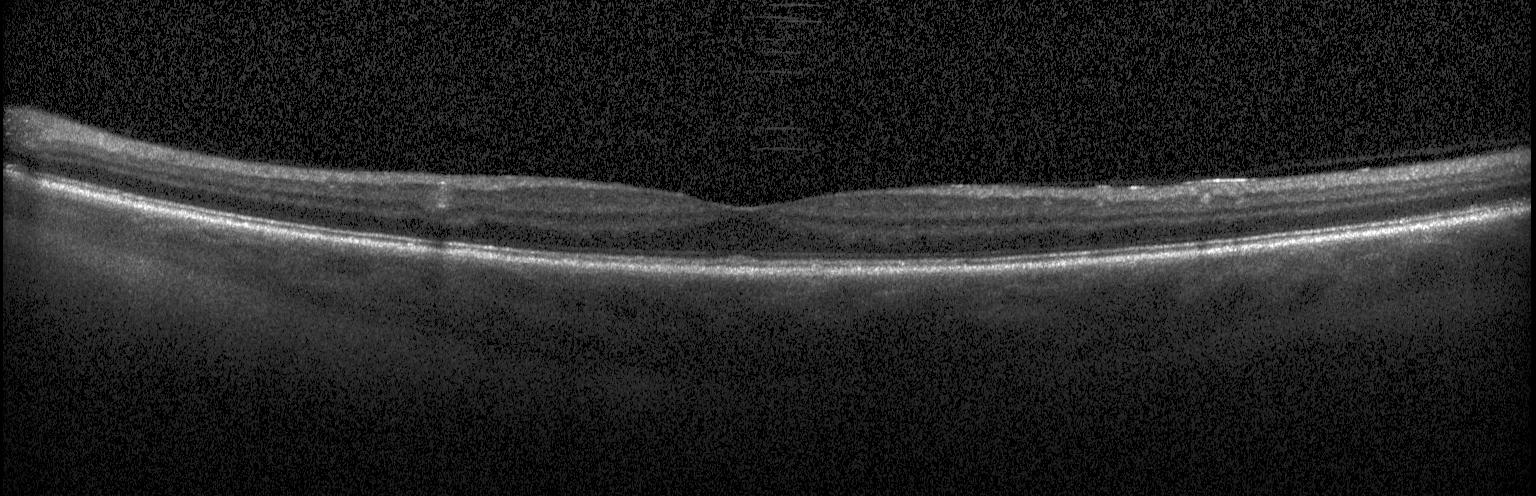
Finding: no evidence of choroidal neovascularization, diabetic macular edema, or drusen.